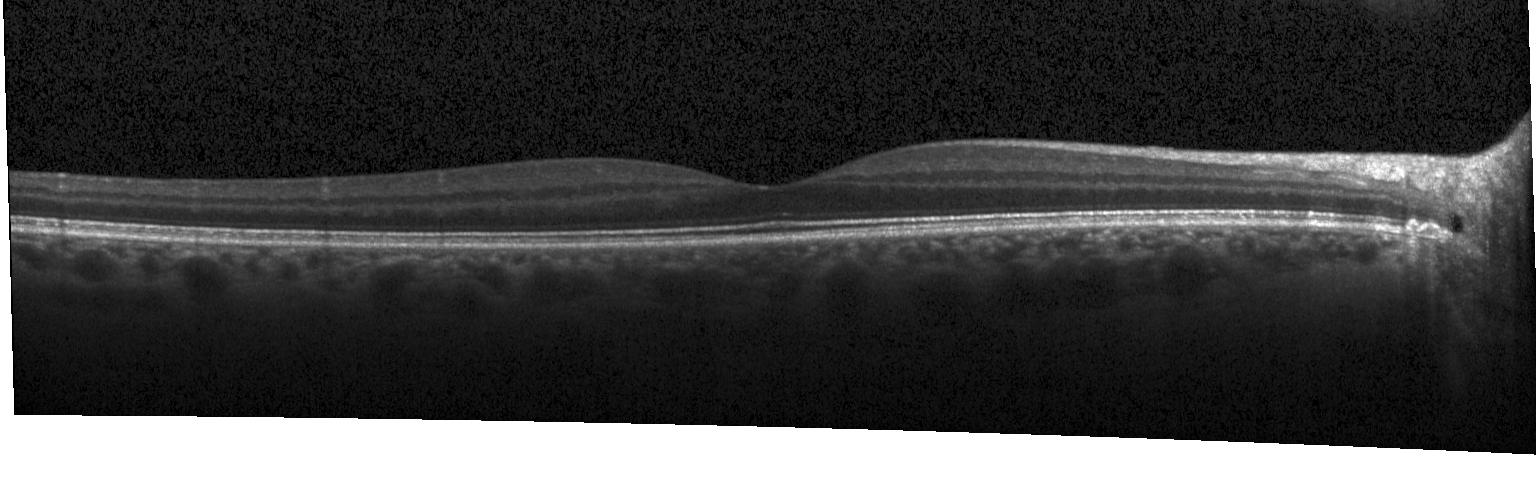

OCT B-scan
Diagnosis: no evidence of choroidal neovascularization, diabetic macular edema, or drusen.